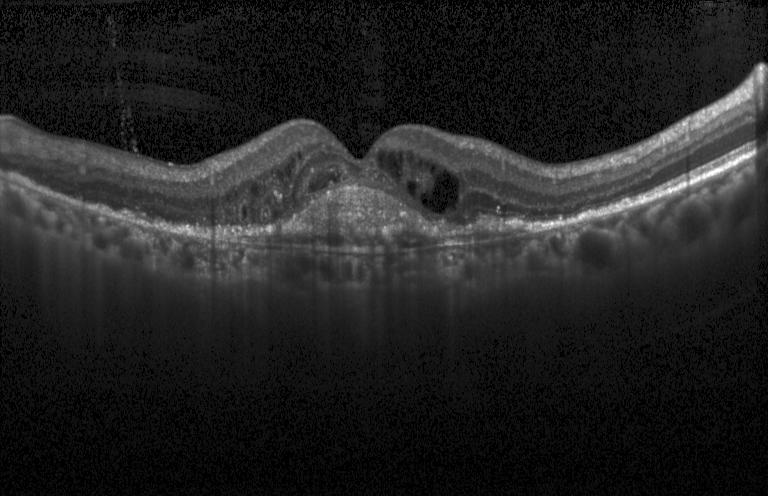
Macular OCT: choroidal neovascularization.